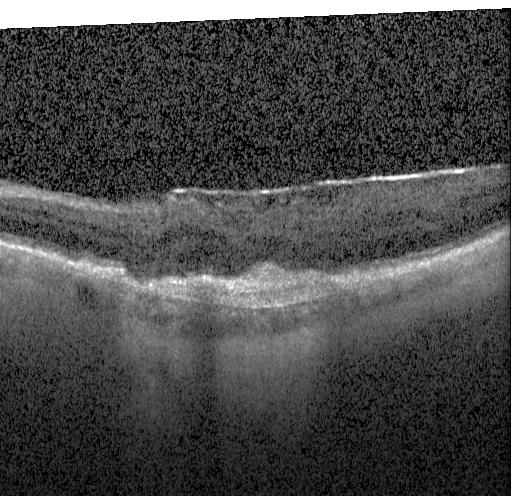 This B-scan demonstrates a choroidal neovascular membrane.